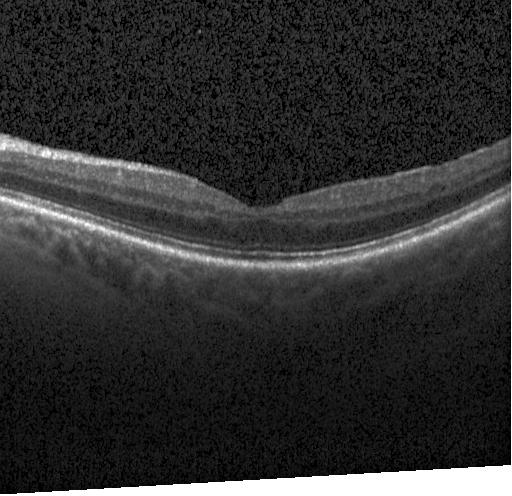

Dx: no CNV, no DME, and no drusen.